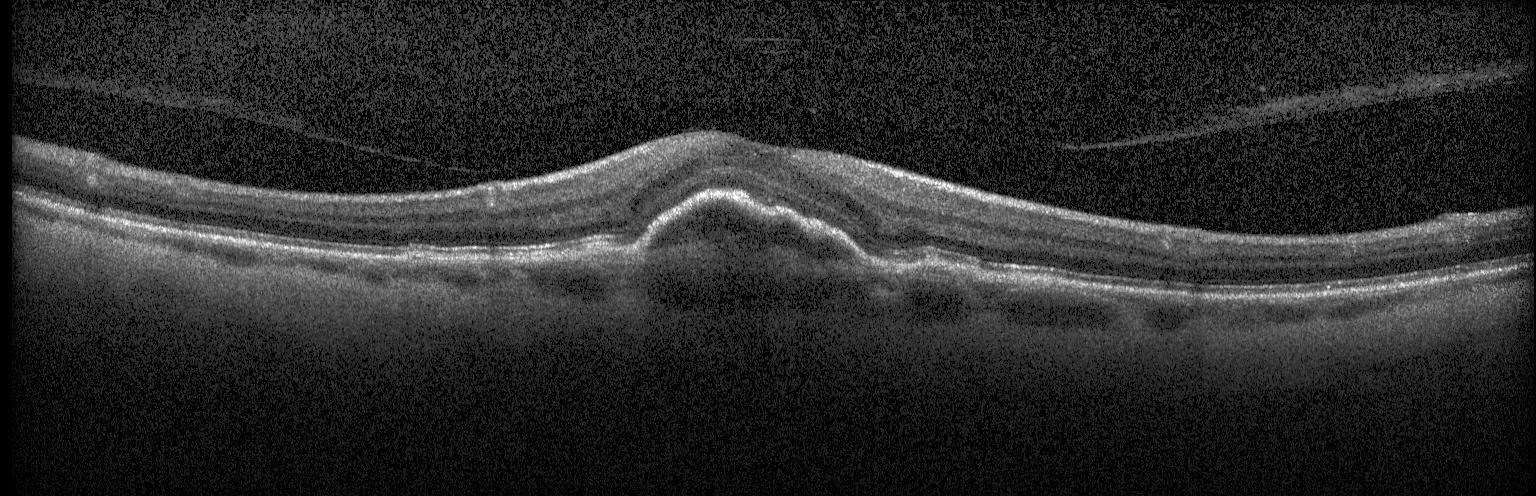 Retinal OCT B-scan, centered on the fovea
Diagnosis: a choroidal neovascular membrane.